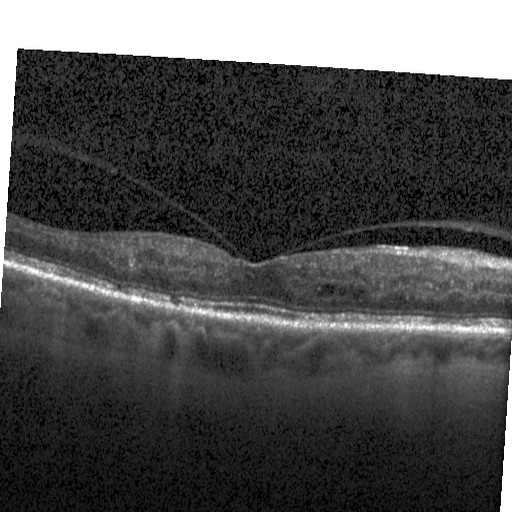

Optical coherence tomography B-scan
Impression: DME.